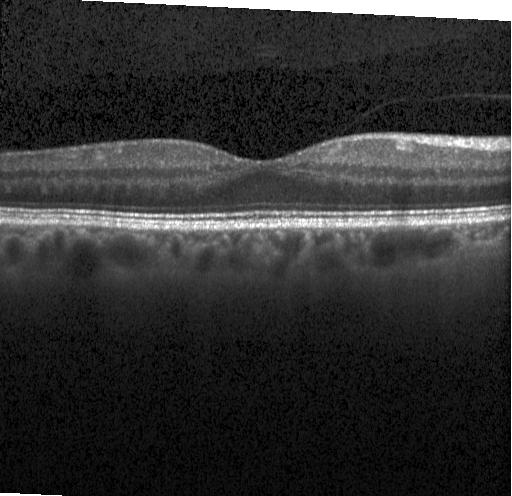
SD-OCT. Optical coherence tomography B-scan. Horizontal scan through the fovea — Dx: no CNV, no DME, and no drusen.